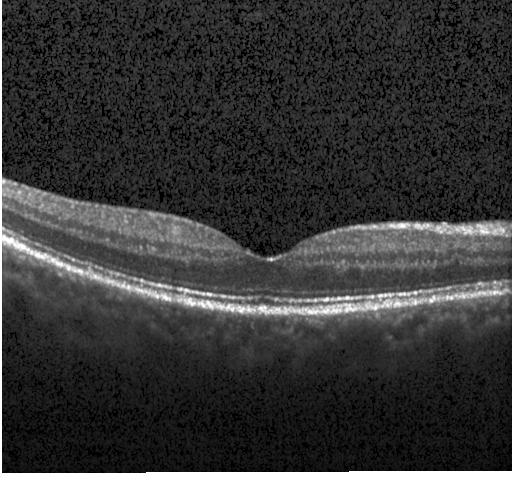 Retinal OCT cross-section.
Assessment: neither choroidal neovascularization, diabetic macular edema, nor drusen.